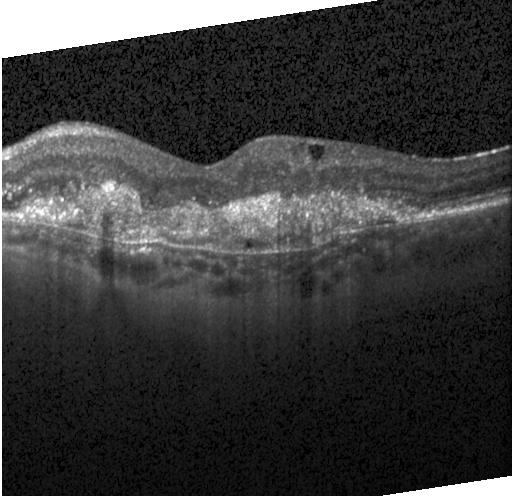

Finding: a choroidal neovascular membrane.